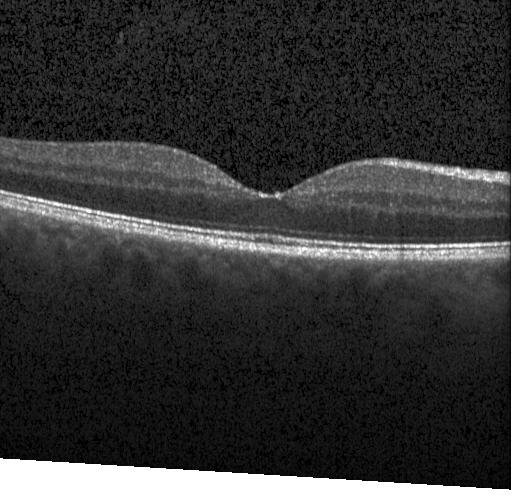
Through the macula. Retinal OCT B-scan. Heidelberg Spectralis OCT system. Spectral-domain optical coherence tomography. Diagnosis: neither choroidal neovascularization, diabetic macular edema, nor drusen.